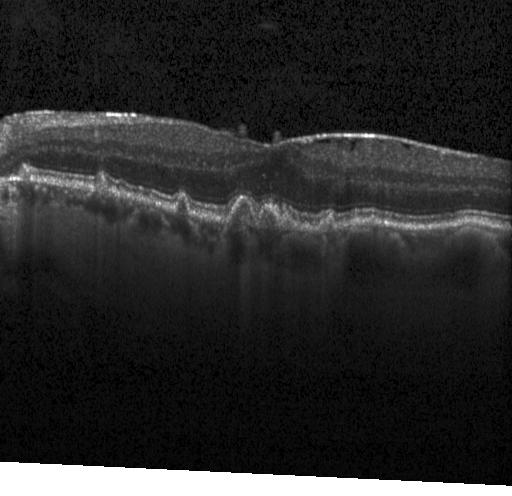
OCT B-scan · spectral-domain optical coherence tomography · through the macula · Heidelberg Spectralis OCT system. The scan shows sub-RPE drusenoid deposits.